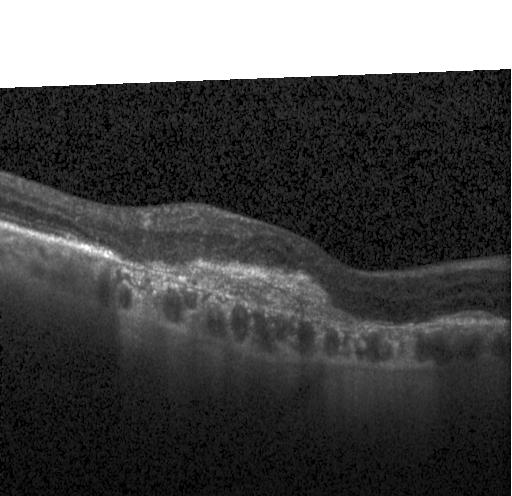
Optical coherence tomography B-scan, centered on the fovea, spectral-domain optical coherence tomography
Diagnosis: CNV.